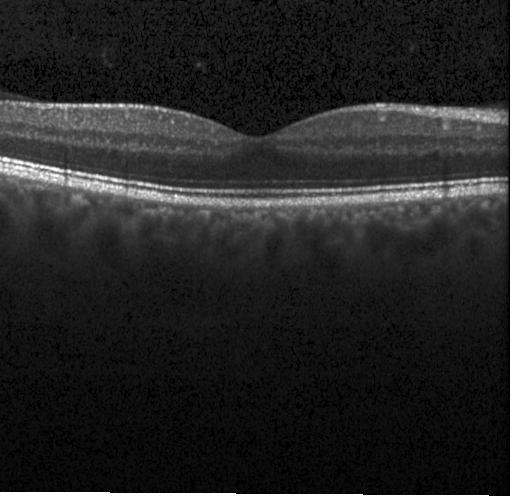

Retinal OCT B-scan. Spectral-domain optical coherence tomography — No evidence of CNV, DME, or drusen.